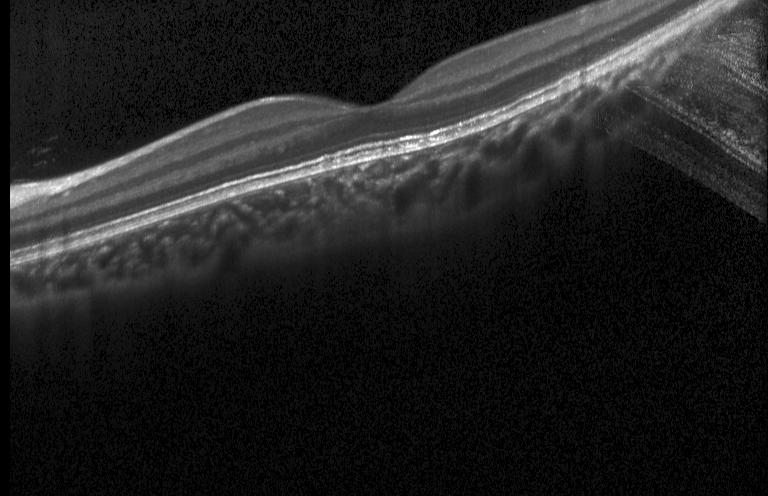
Neither CNV, DME, nor drusen.